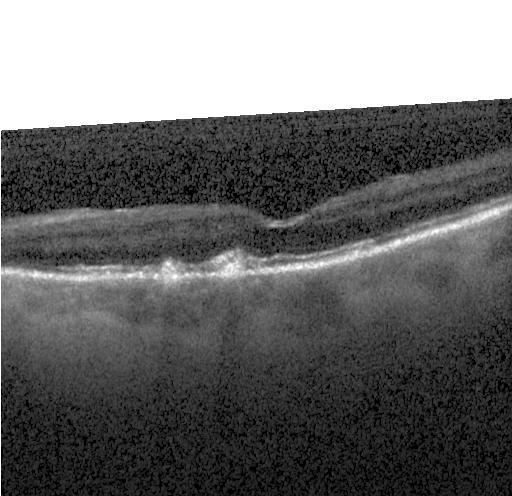

Heidelberg Spectralis. Fovea-centered. Optical coherence tomography B-scan. Spectral-domain OCT. Diagnosis: choroidal neovascularization (CNV).